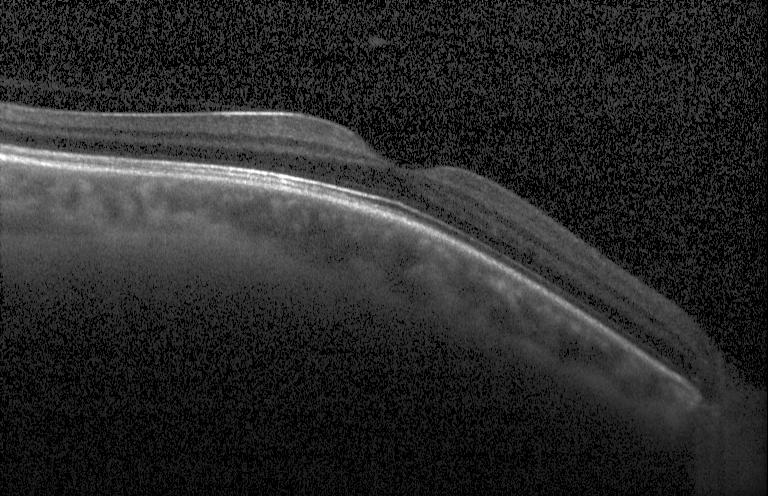 SD-OCT · acquired on a Heidelberg Spectralis · horizontal scan through the fovea · OCT B-scan.
No choroidal neovascularization, no diabetic macular edema, and no drusen.